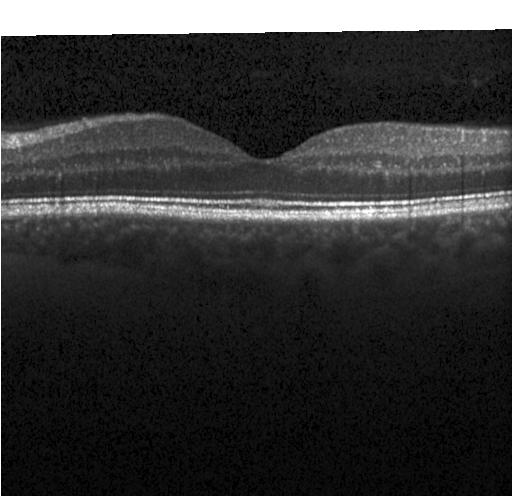
Diagnosis: no CNV, DME, or drusen.